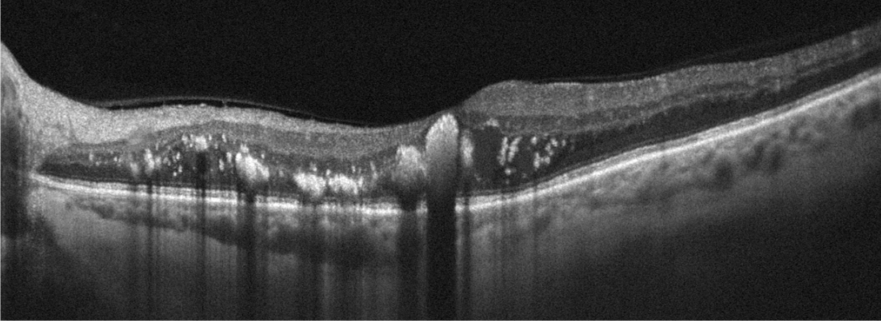 Instrument: Optovue Avanti RTVue XR; OCT B-scan; through the macula.
Finding: DME.